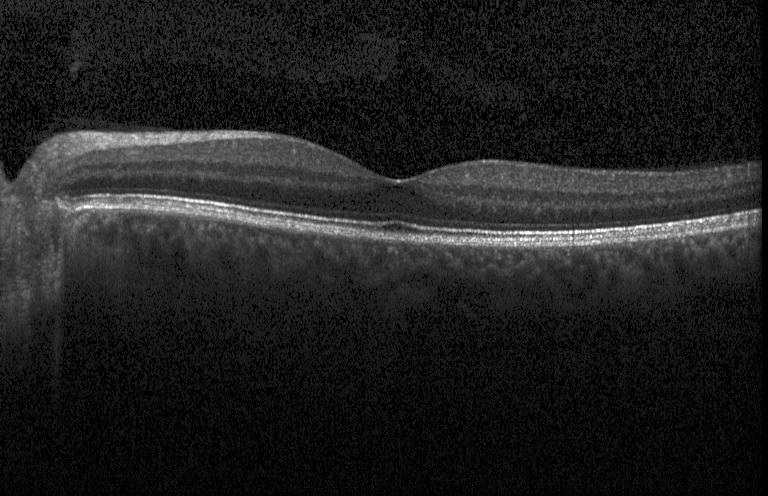

SD-OCT; through the macula; Heidelberg Spectralis; retinal OCT cross-section.
Dx: no CNV, no DME, and no drusen.